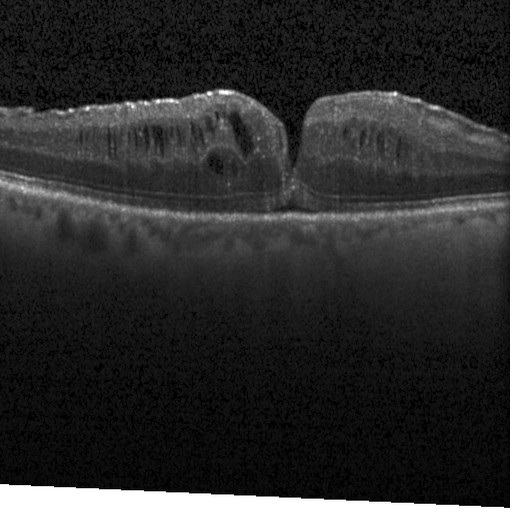

Heidelberg Spectralis OCT system; OCT B-scan
Diagnosis: DME.